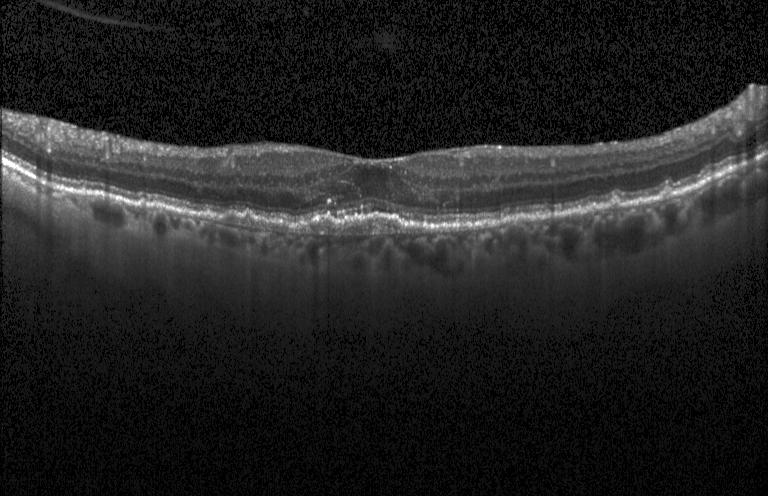
Acquired on a Heidelberg Spectralis · spectral-domain OCT · retinal OCT cross-section
The scan shows CNV.